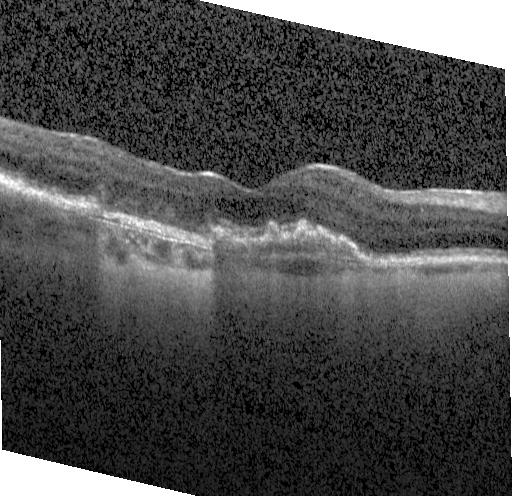
Optical coherence tomography scan — Macular OCT: a choroidal neovascular membrane.